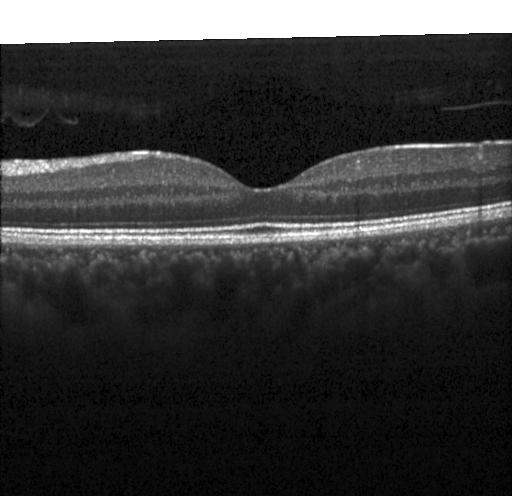
Optical coherence tomography scan. Finding: neither choroidal neovascularization, diabetic macular edema, nor drusen.